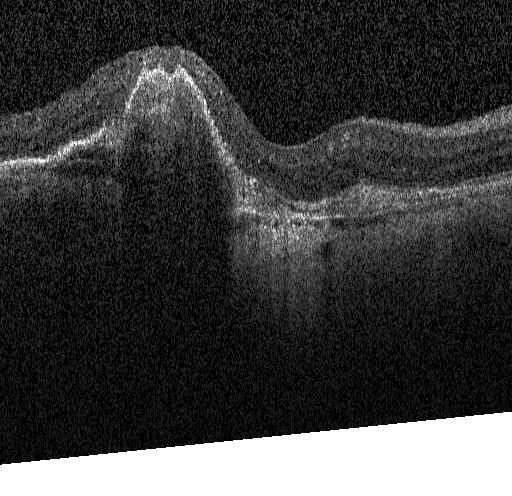

Spectral-domain optical coherence tomography · OCT line scan — A choroidal neovascular membrane.